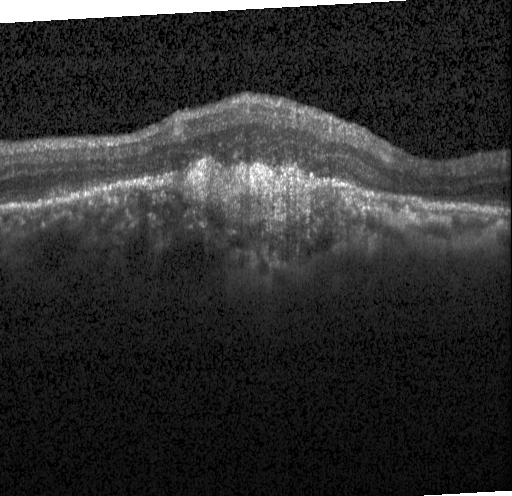 Retinal OCT cross-section.
Impression: a choroidal neovascular membrane.